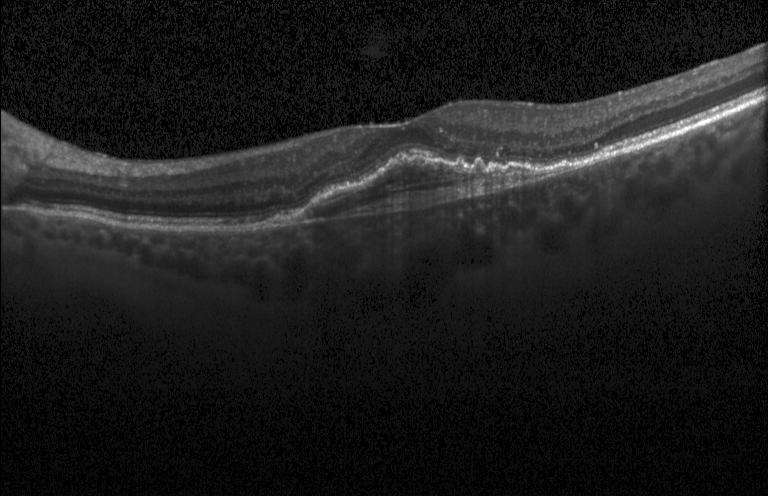
Optical coherence tomography scan
Impression: a choroidal neovascular membrane.